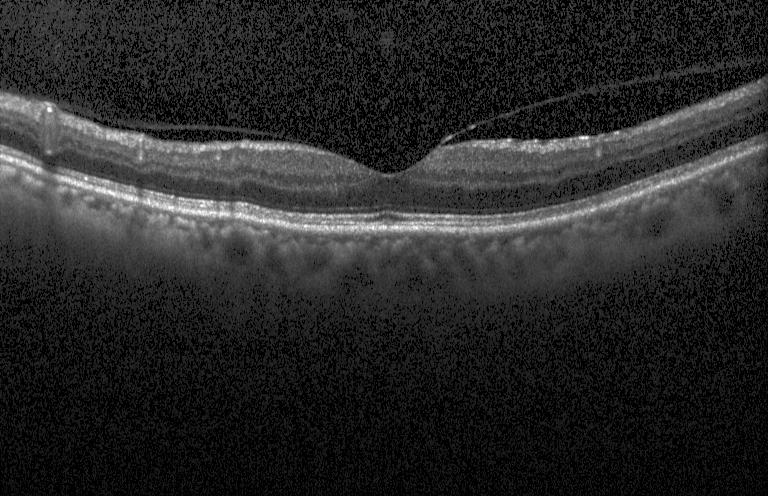

Finding: no CNV, DME, or drusen.